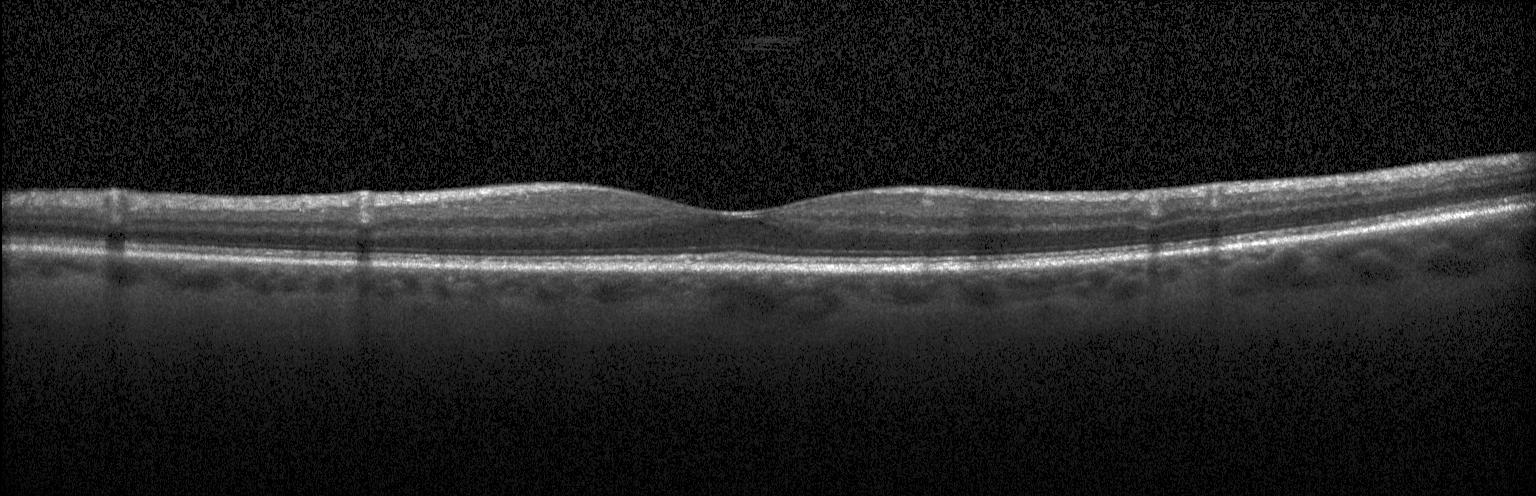
Spectral-domain OCT · OCT line scan · horizontal scan through the fovea. The scan shows neither choroidal neovascularization, diabetic macular edema, nor drusen.